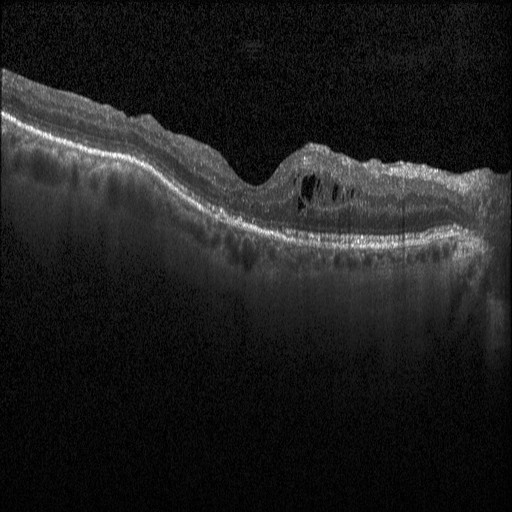
Macular OCT: DME.